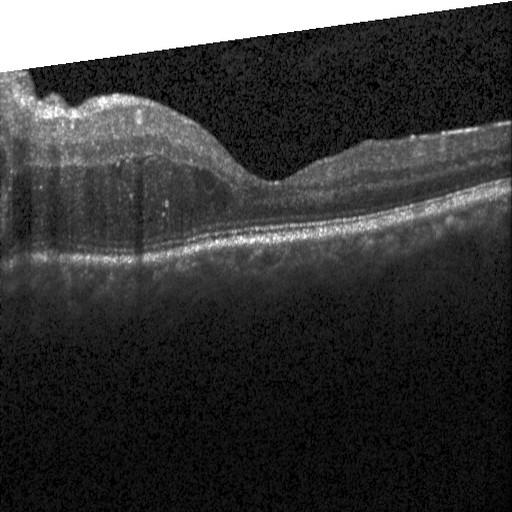

OCT scan showing diabetic macular edema.